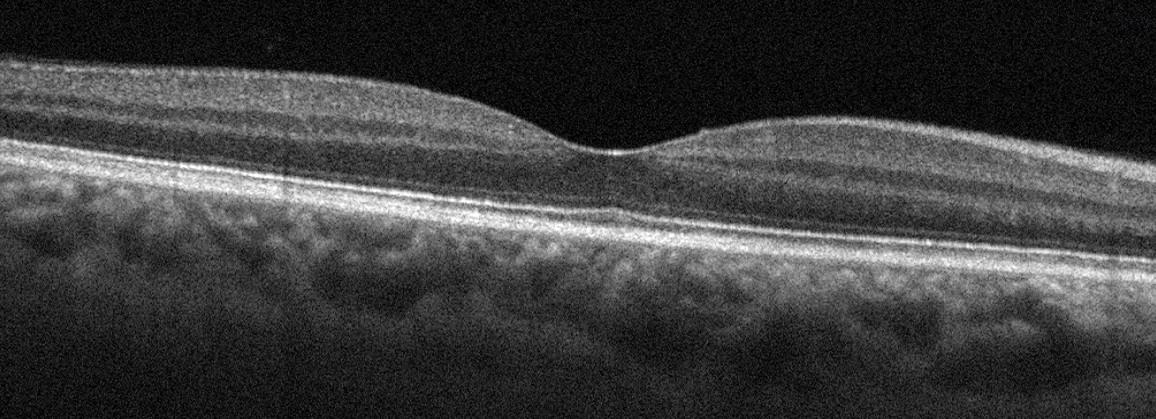
Retinal OCT cross-section. This B-scan demonstrates no evidence of AMD, DME, ERM, RAO, RVO, or VID.